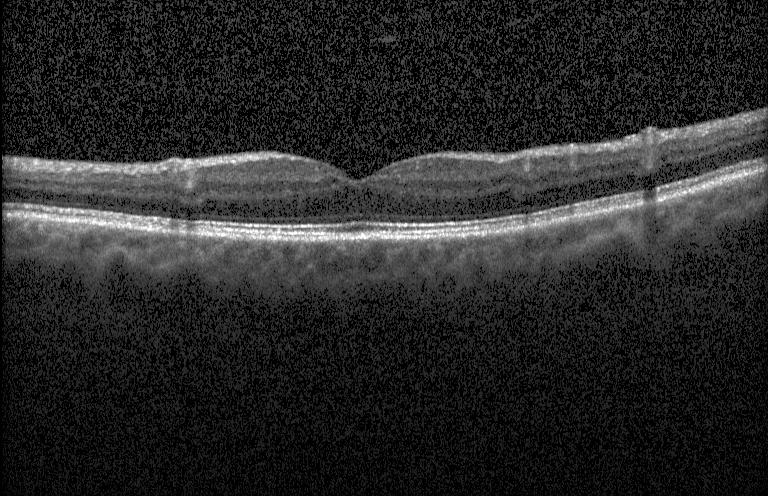
Heidelberg Spectralis OCT system · OCT B-scan · SD-OCT. The scan shows neither choroidal neovascularization, diabetic macular edema, nor drusen.